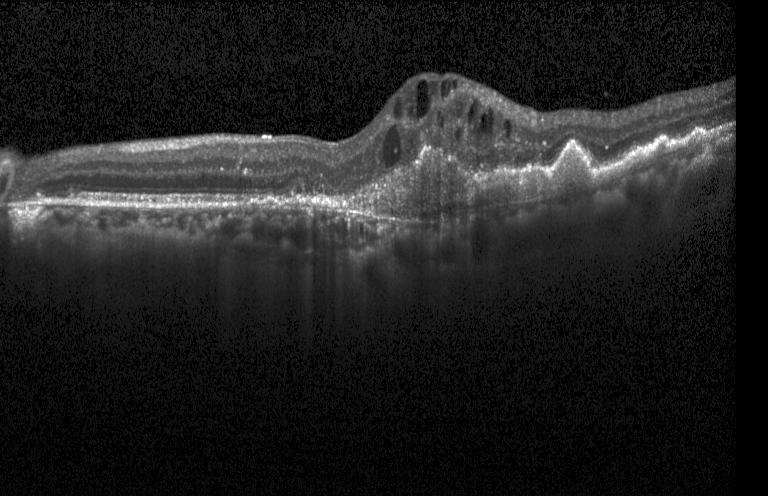 Optical coherence tomography B-scan
Diagnosis: choroidal neovascularization.